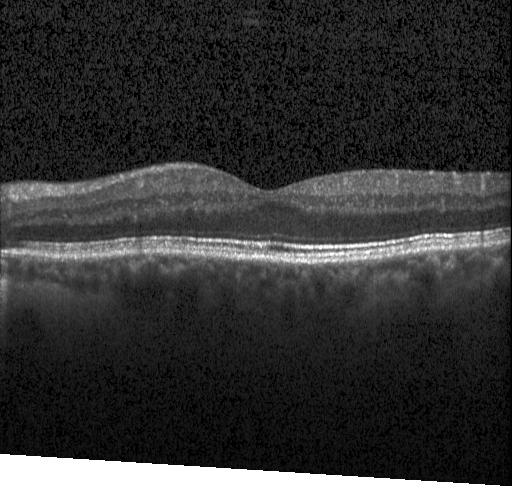
Horizontal scan through the fovea. Optical coherence tomography B-scan. Instrument: Heidelberg Spectralis. Spectral-domain OCT. Dx: neither CNV, DME, nor drusen.